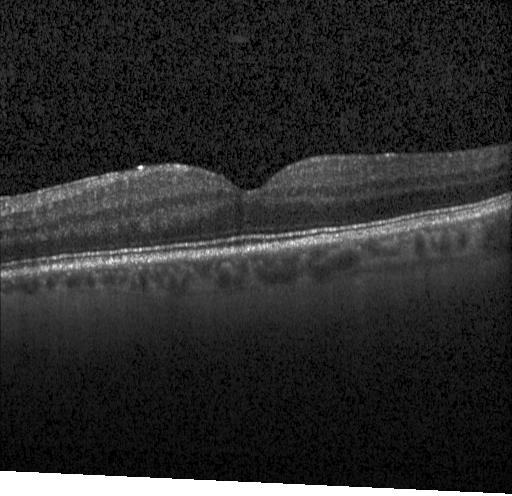

OCT finding: no CNV, DME, or drusen.